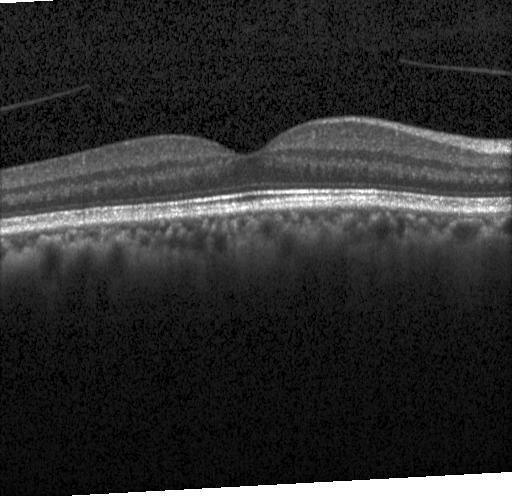

SD-OCT; OCT line scan; centered on the fovea.
Finding: no choroidal neovascularization, diabetic macular edema, or drusen.